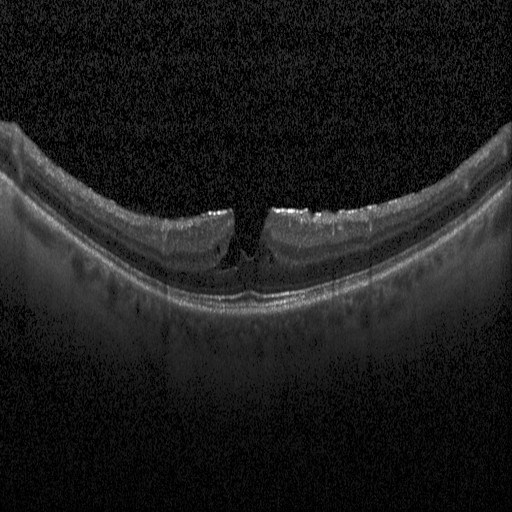
Retinal OCT cross-section showing DME.